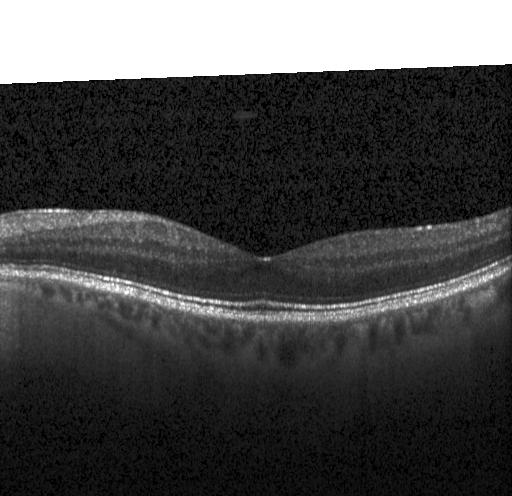 OCT B-scan — Finding: no choroidal neovascularization, no diabetic macular edema, and no drusen.